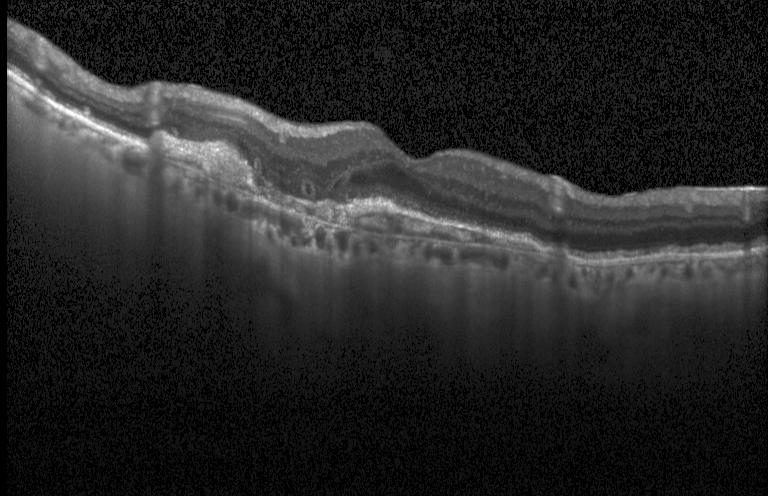
Retinal OCT cross-section.
OCT finding: CNV.